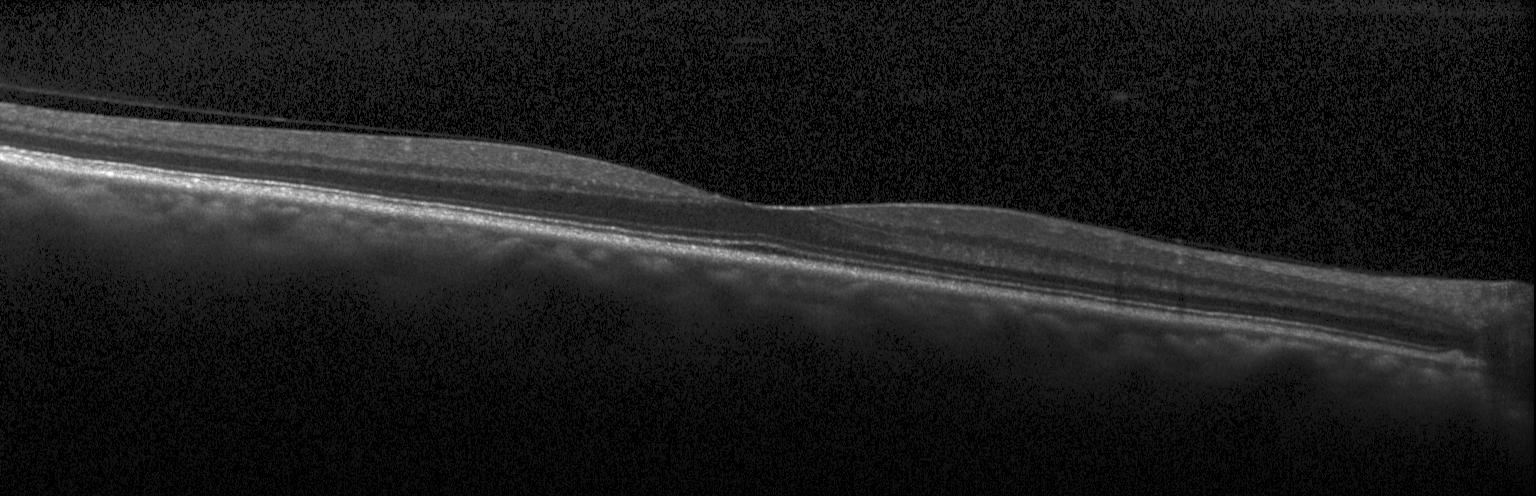 Diagnosis: neither CNV, DME, nor drusen.